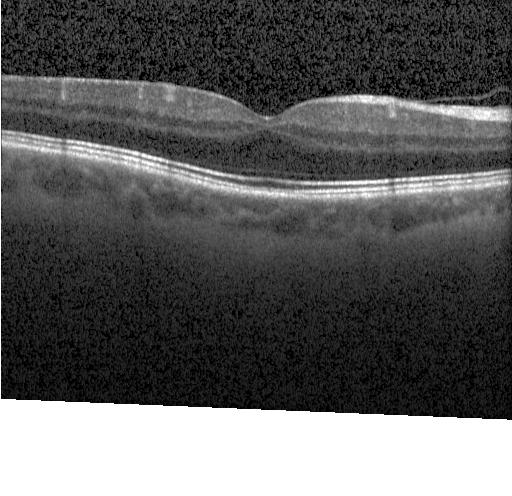
OCT line scan. Assessment: no choroidal neovascularization, diabetic macular edema, or drusen.